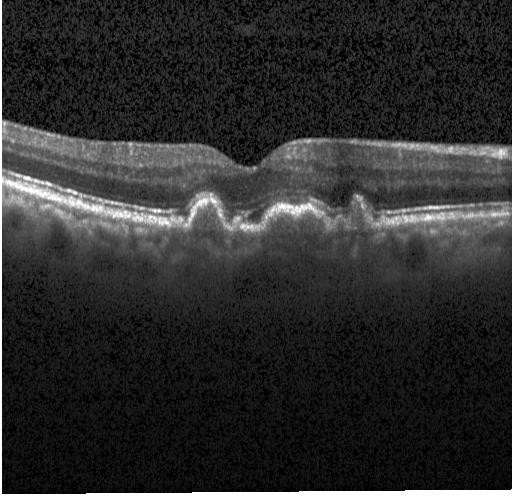 Spectral-domain optical coherence tomography, OCT line scan, fovea-centered
Finding: sub-RPE drusenoid deposits.